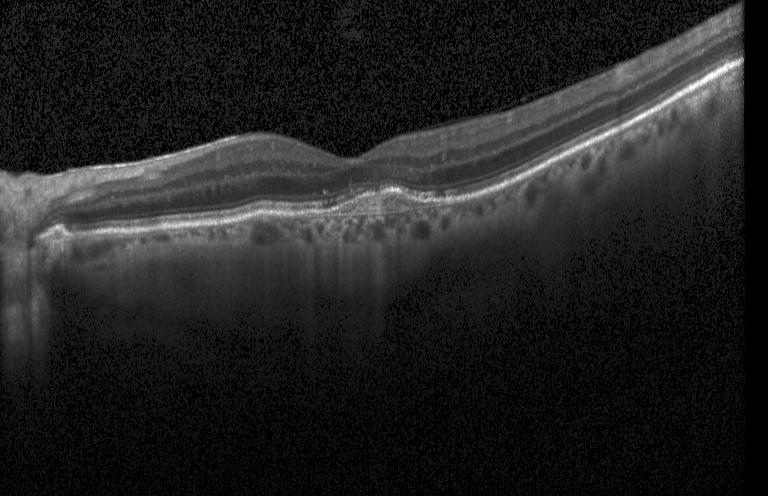 OCT B-scan · acquired on a Heidelberg Spectralis
Finding: choroidal neovascularization (CNV).